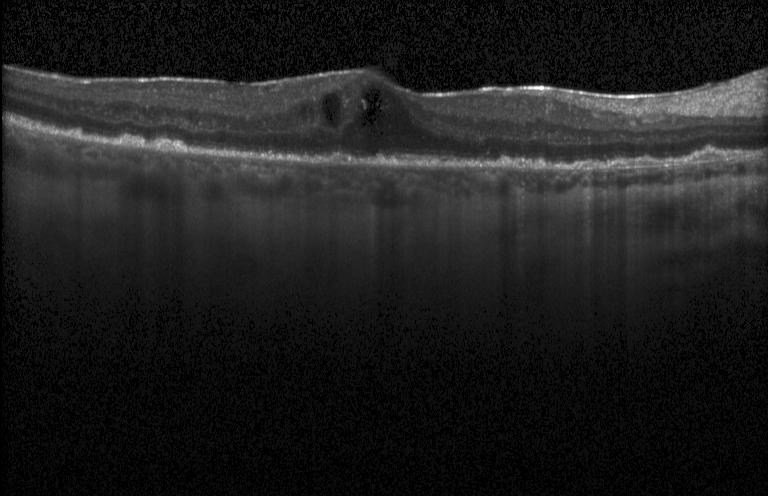
Retinal OCT cross-section. Assessment: diabetic macular edema.